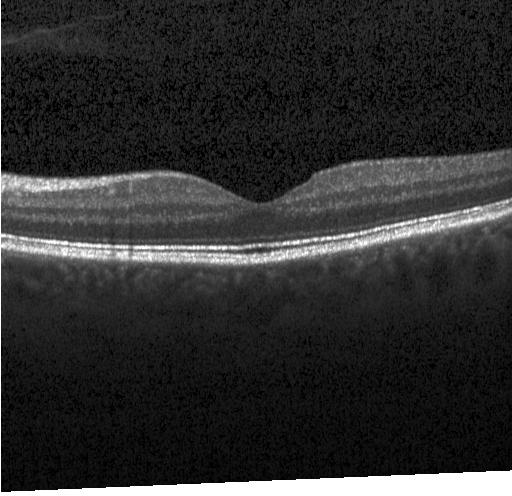
Diagnosis: no CNV, no DME, and no drusen.